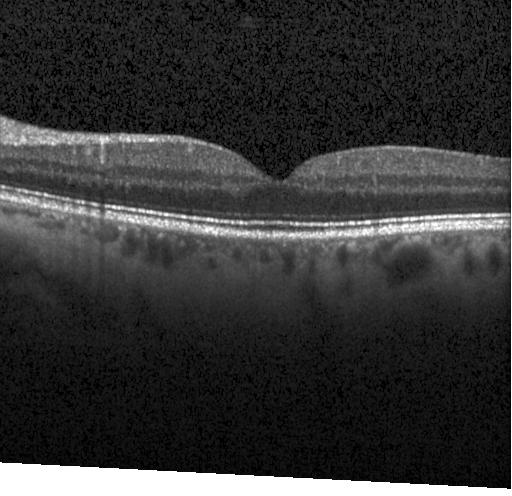 SD-OCT. Acquired on a Heidelberg Spectralis. Retinal OCT B-scan. Fovea-centered — The scan shows no choroidal neovascularization, diabetic macular edema, or drusen.